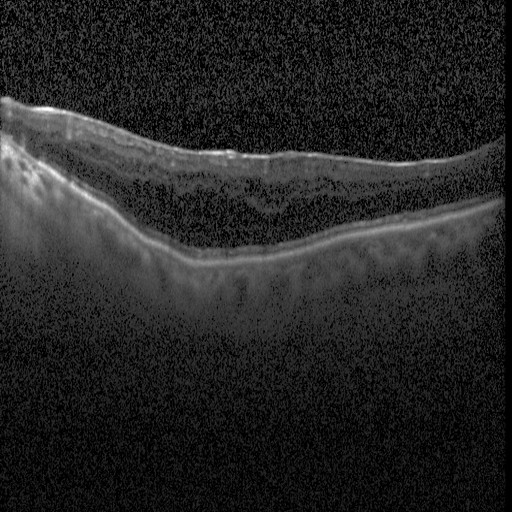 SD-OCT; retinal OCT B-scan; fovea-centered.
Diagnosis: diabetic macular edema (DME).